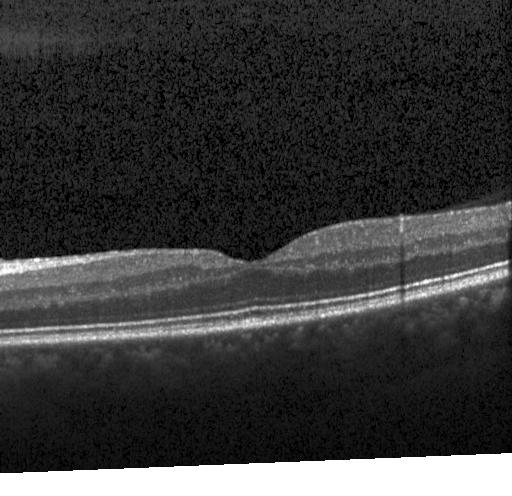 Fovea-centered. OCT line scan.
The scan shows no choroidal neovascularization, diabetic macular edema, or drusen.